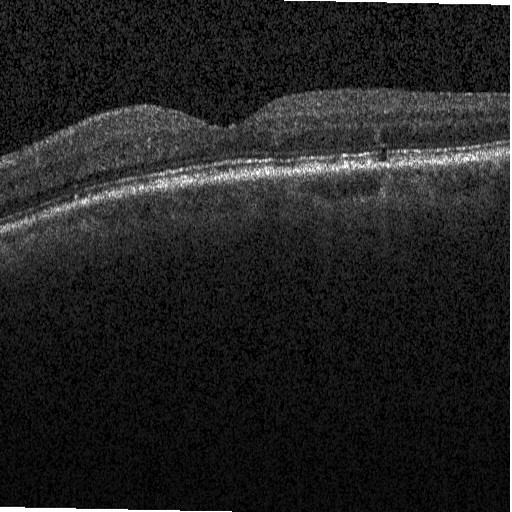
Horizontal scan through the fovea. OCT B-scan. Impression: diabetic macular edema.